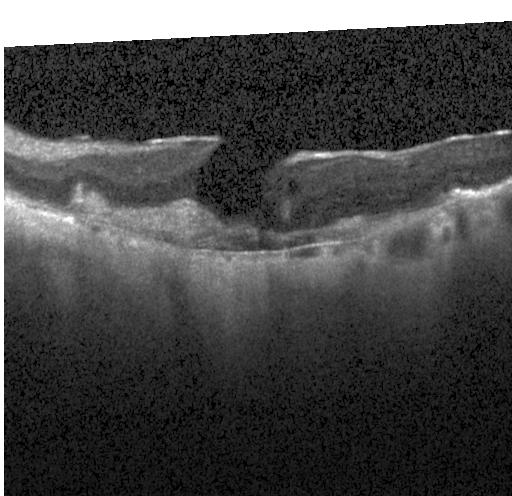
Acquired on a Heidelberg Spectralis. Optical coherence tomography scan. Macular scan
The scan shows a choroidal neovascular membrane.